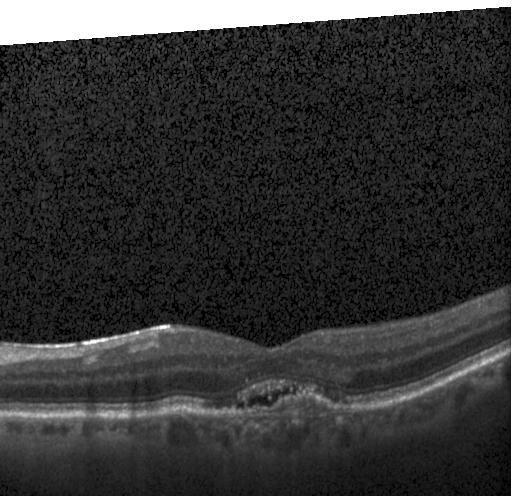 Finding: CNV.